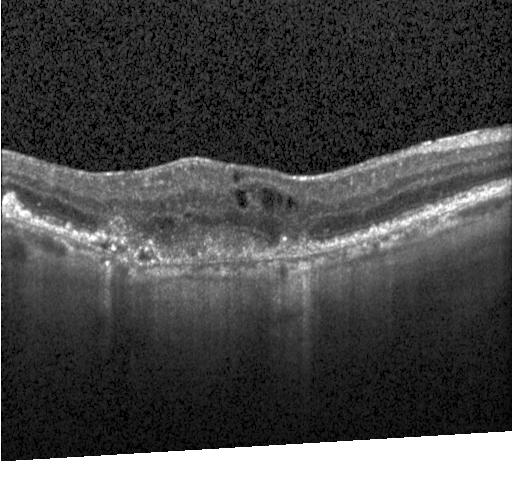

Optical coherence tomography scan
Assessment: a choroidal neovascular membrane.